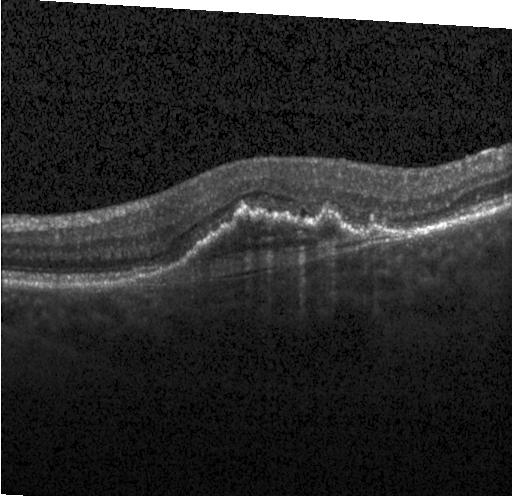

Retinal OCT B-scan.
Finding: a choroidal neovascular membrane.